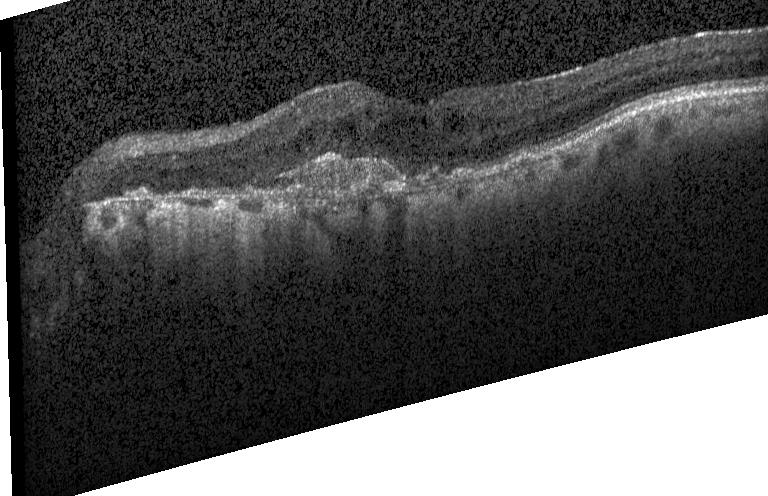

Finding: choroidal neovascularization (CNV).